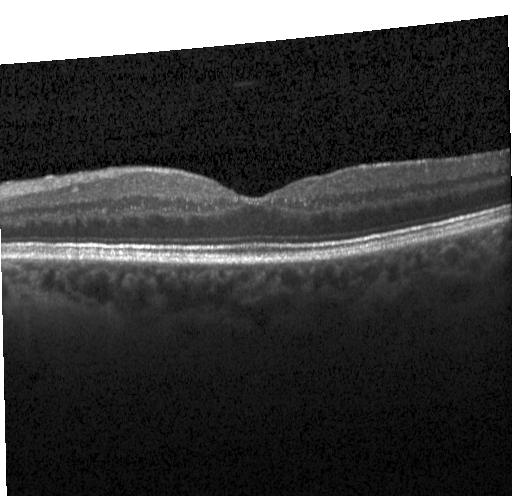

Macular scan · OCT line scan · instrument: Heidelberg Spectralis · spectral-domain optical coherence tomography — Neither CNV, DME, nor drusen.